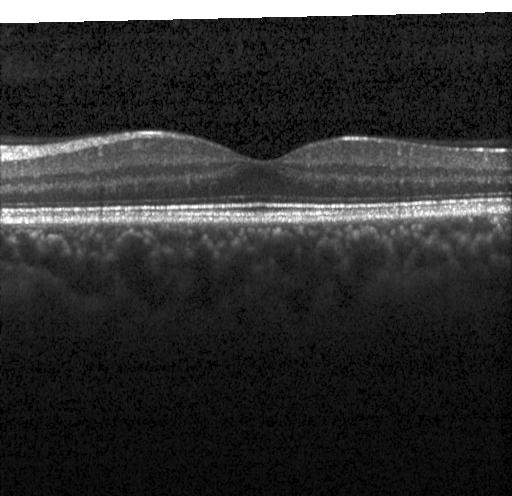 OCT line scan; SD-OCT; acquired on a Heidelberg Spectralis. Diagnosis: no choroidal neovascularization, diabetic macular edema, or drusen.